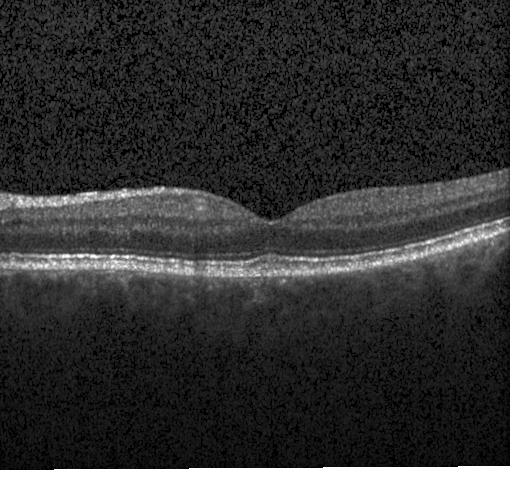 This B-scan demonstrates no choroidal neovascularization, no diabetic macular edema, and no drusen.